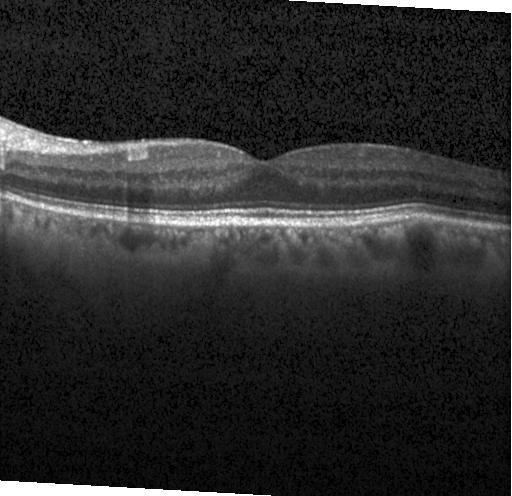
Macular OCT demonstrating no evidence of choroidal neovascularization, diabetic macular edema, or drusen.